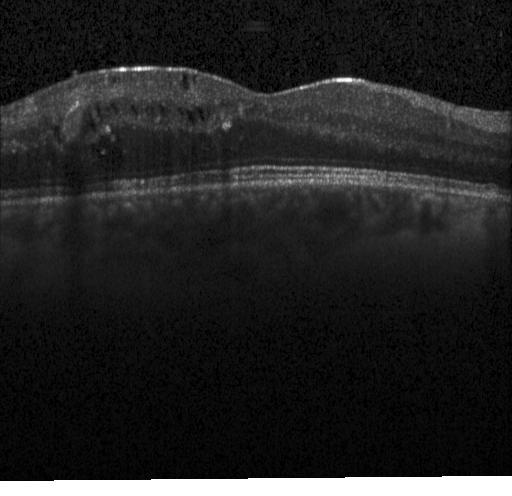

Acquired on a Heidelberg Spectralis. Retinal OCT B-scan. Centered on the fovea. Spectral-domain optical coherence tomography.
Dx: diabetic macular edema.